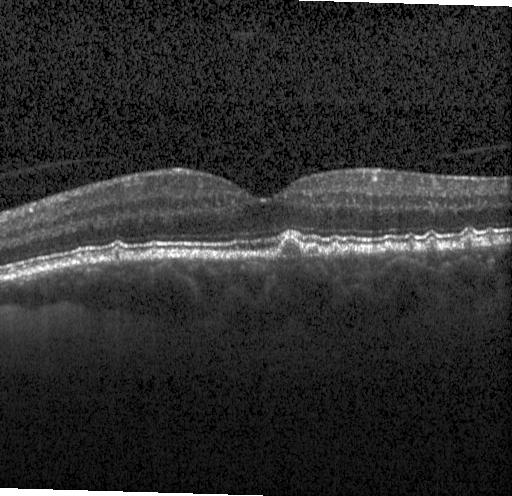 Impression: sub-RPE drusenoid deposits.